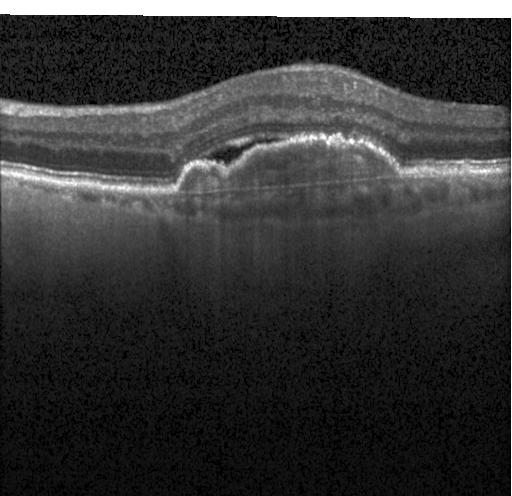
This B-scan demonstrates choroidal neovascularization (CNV).